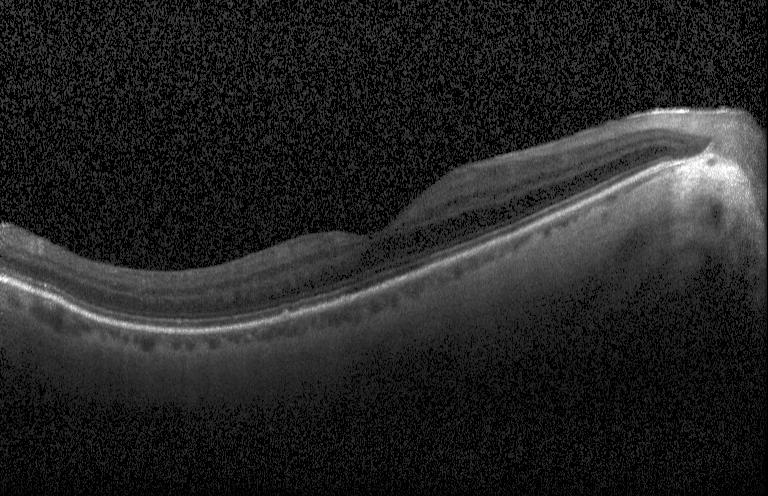
Retinal OCT B-scan.
Diagnosis: sub-RPE drusenoid deposits.